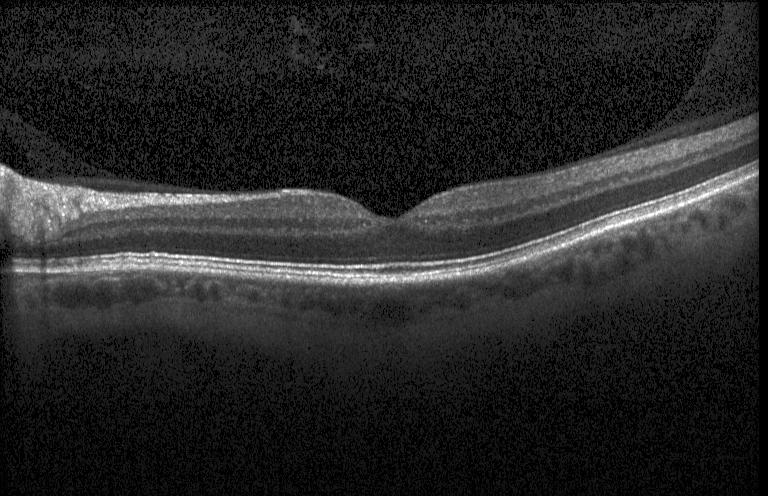

Heidelberg Spectralis OCT system. Retinal OCT cross-section. Macular scan — Impression: no evidence of choroidal neovascularization, diabetic macular edema, or drusen.